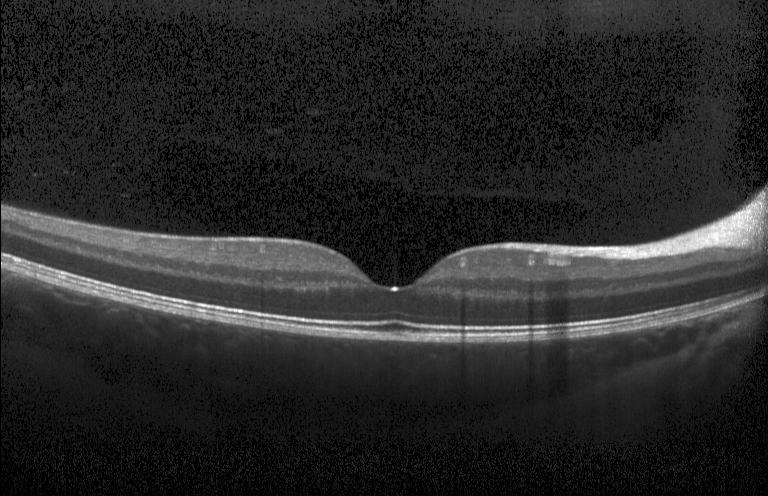 Impression: no choroidal neovascularization, no diabetic macular edema, and no drusen.